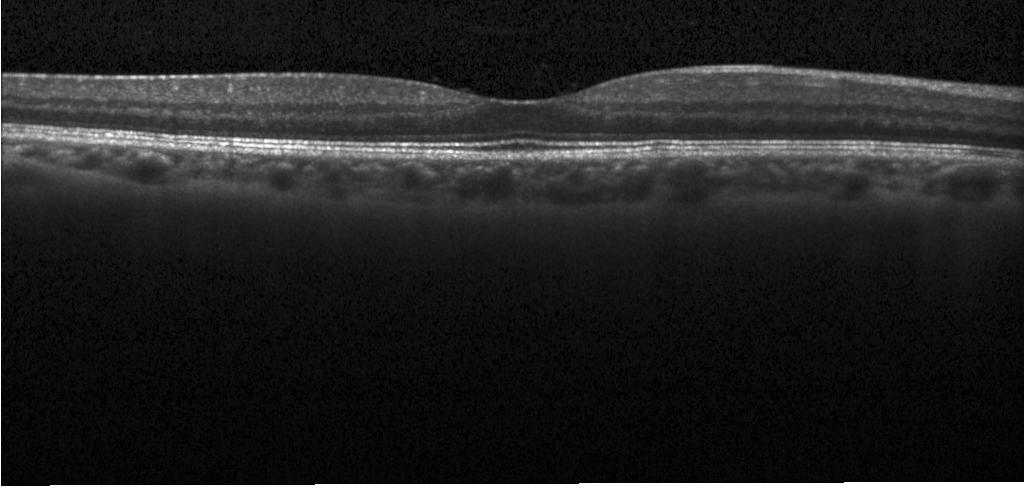
Spectral-domain optical coherence tomography; OCT line scan; centered on the fovea
Diagnosis: no choroidal neovascularization, no diabetic macular edema, and no drusen.